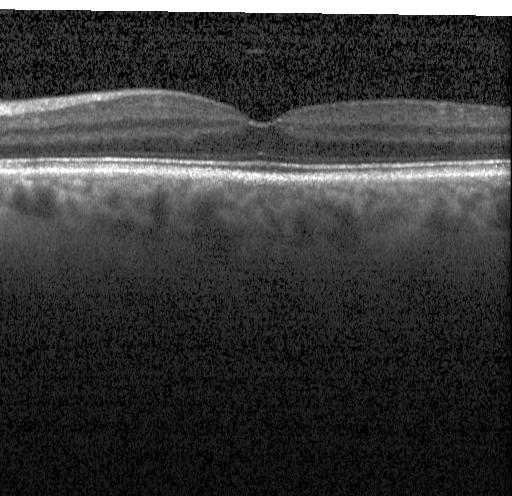 Spectral-domain OCT · through the macula · Heidelberg Spectralis · optical coherence tomography scan. Finding: no choroidal neovascularization, no diabetic macular edema, and no drusen.